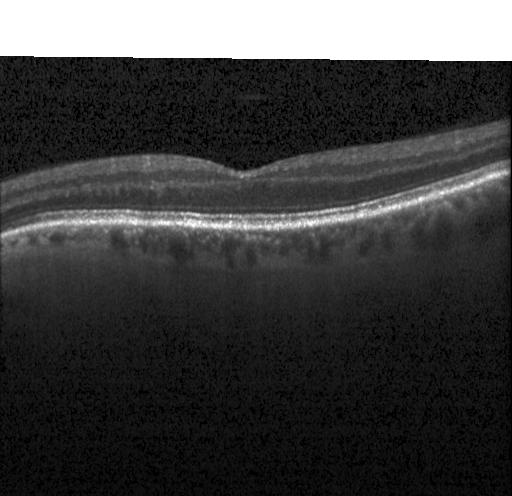
Retinal OCT B-scan
This B-scan demonstrates no evidence of choroidal neovascularization, diabetic macular edema, or drusen.